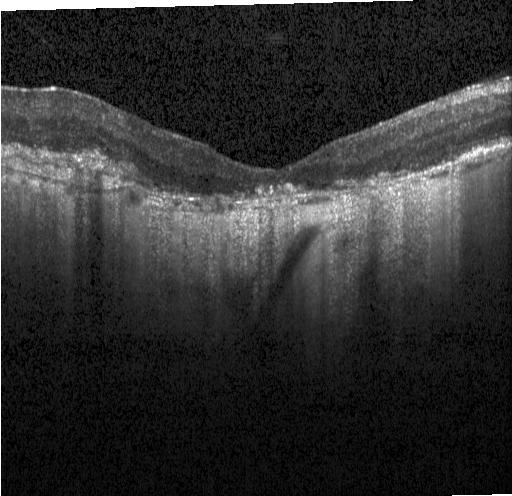
Assessment: choroidal neovascularization (CNV).